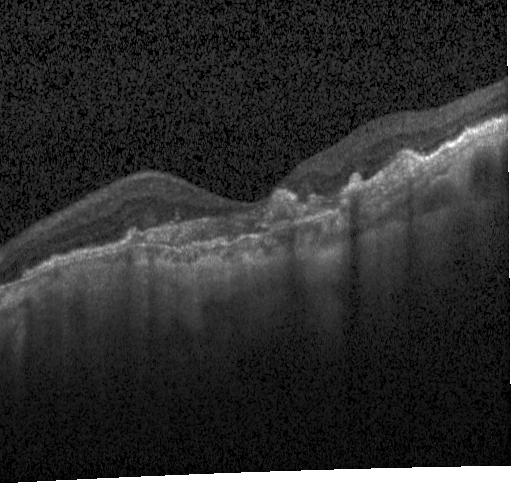

Fovea-centered. Optical coherence tomography B-scan. SD-OCT.
A choroidal neovascular membrane.